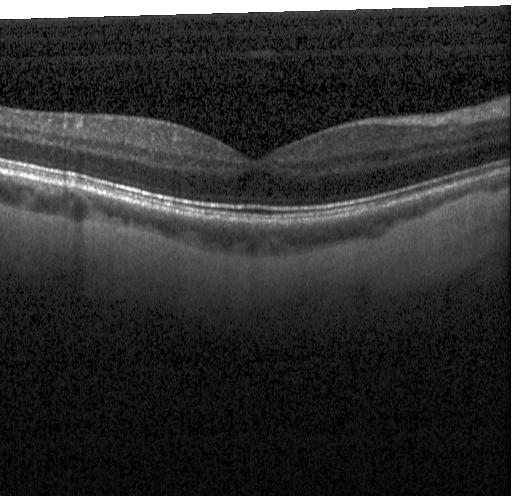
Finding: neither choroidal neovascularization, diabetic macular edema, nor drusen.